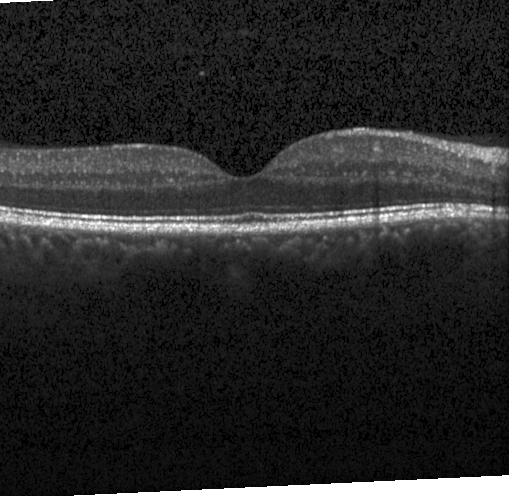
OCT B-scan · spectral-domain optical coherence tomography — Assessment: no evidence of CNV, DME, or drusen.